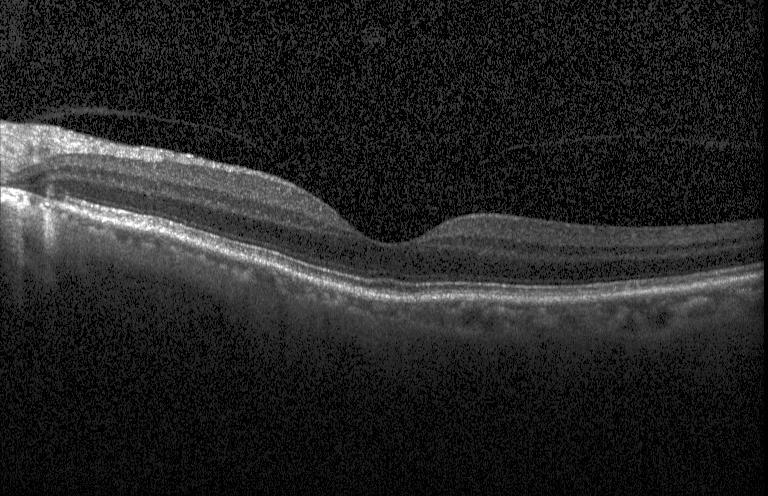

Heidelberg Spectralis OCT system, spectral-domain OCT, optical coherence tomography B-scan, through the macula. Finding: no choroidal neovascularization, diabetic macular edema, or drusen.